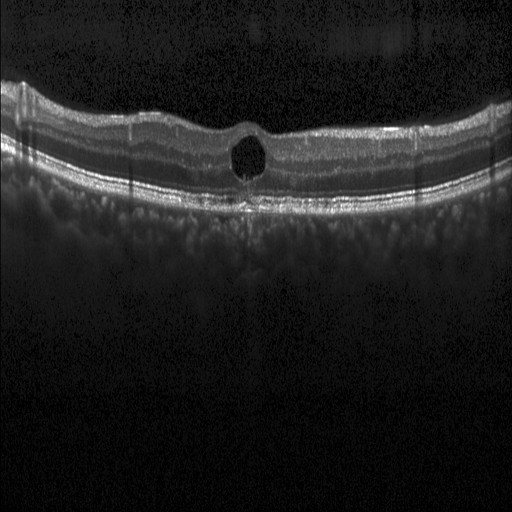 Through the macula. Heidelberg Spectralis. SD-OCT. OCT B-scan
Dx: DME.